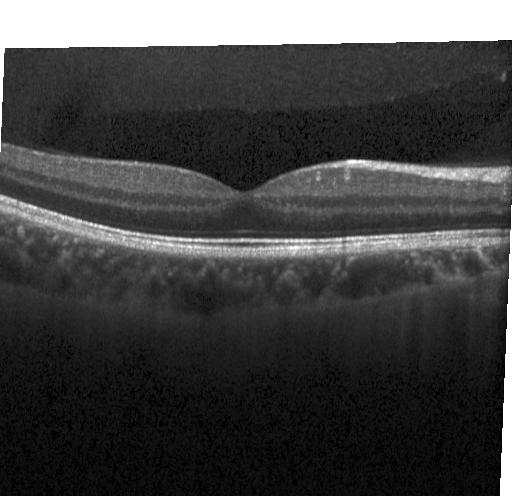 Retinal OCT cross-section — Finding: no choroidal neovascularization, no diabetic macular edema, and no drusen.